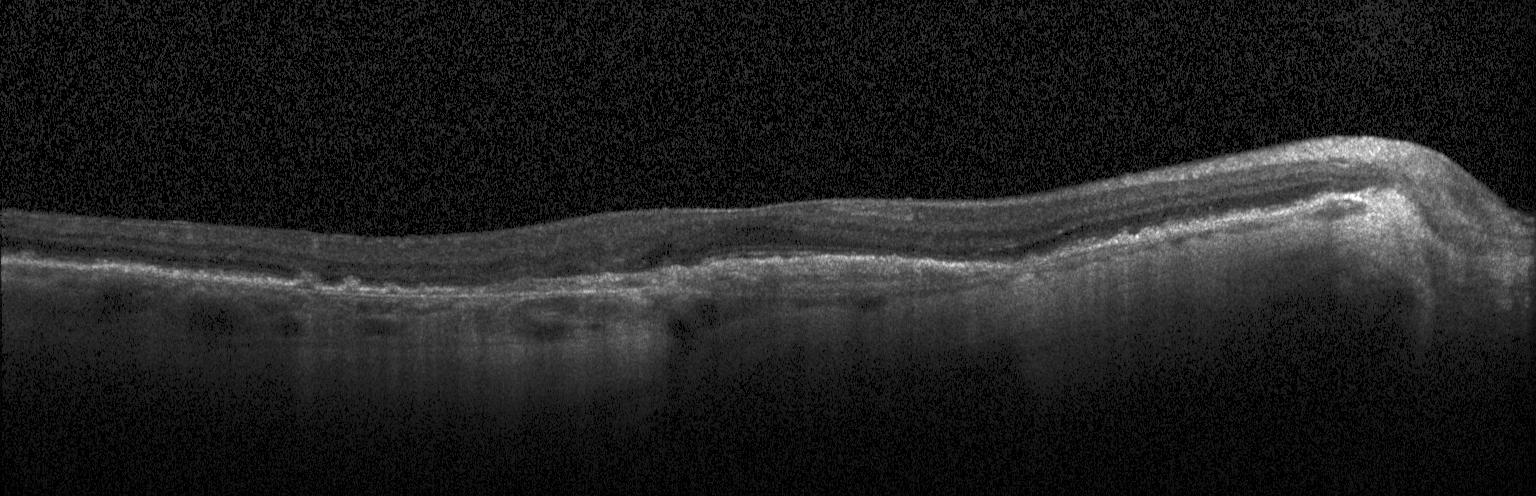 Retinal OCT cross-section showing a choroidal neovascular membrane.